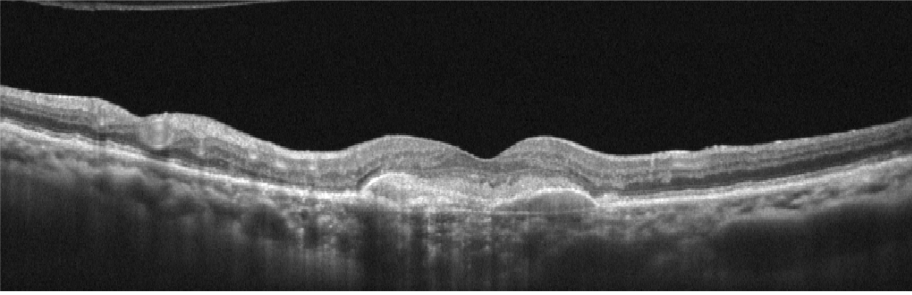 Optical coherence tomography B-scan, acquired on an Optovue Avanti RTVue XR. The scan shows AMD.